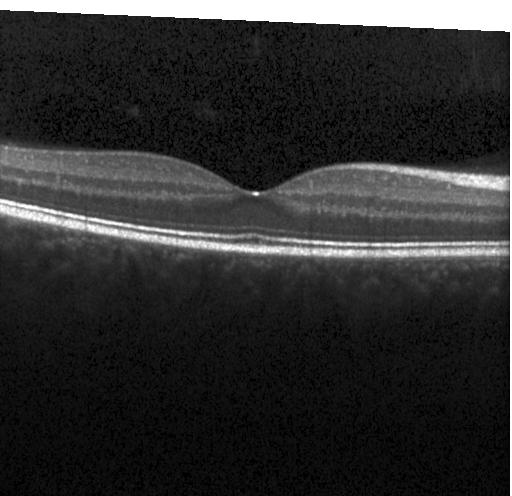

Optical coherence tomography B-scan. This B-scan demonstrates neither choroidal neovascularization, diabetic macular edema, nor drusen.